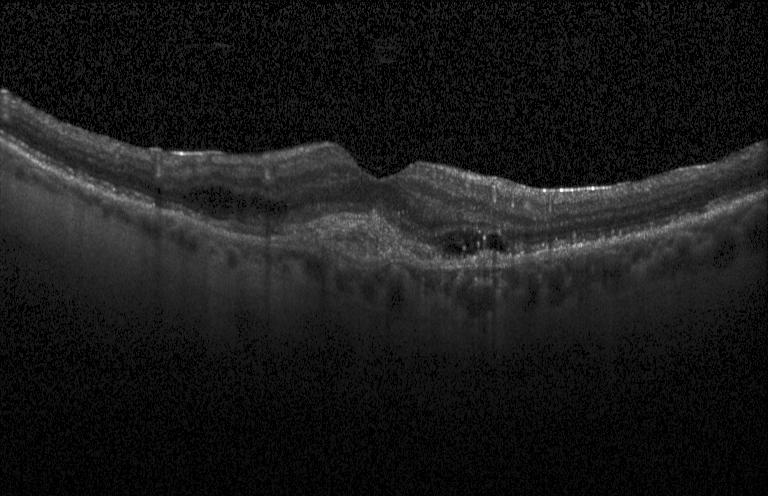

OCT line scan. Instrument: Heidelberg Spectralis. Spectral-domain optical coherence tomography. Fovea-centered
Diagnosis: a choroidal neovascular membrane.